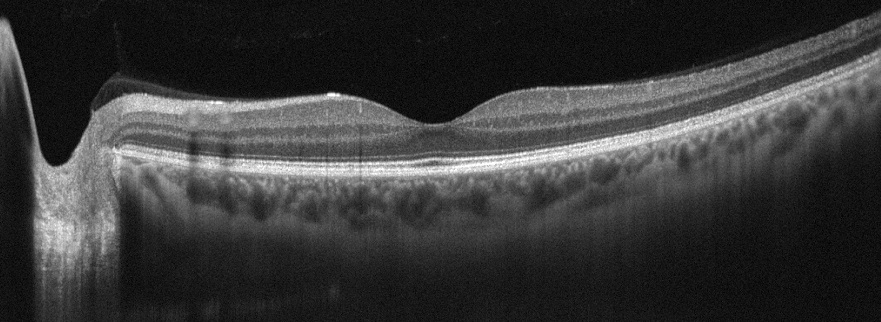 Retinal OCT cross-section; instrument: Optovue Avanti RTVue XR.
Finding: absence of AMD, DME, ERM, RAO, RVO, and vitreomacular interface disease.